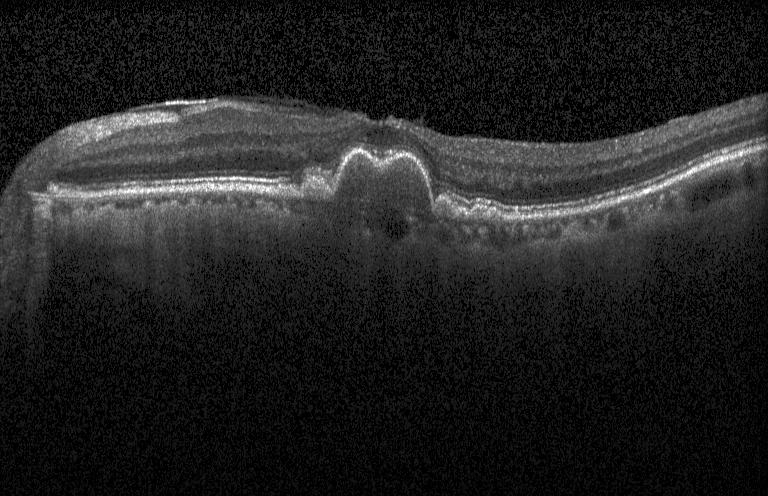 Retinal OCT cross-section.
Dx: a choroidal neovascular membrane.